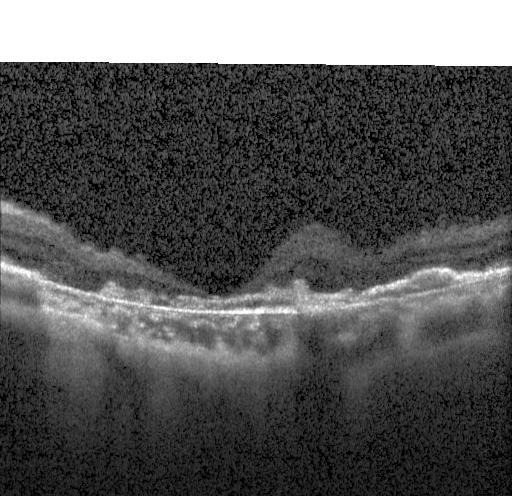
Diagnosis: a choroidal neovascular membrane.